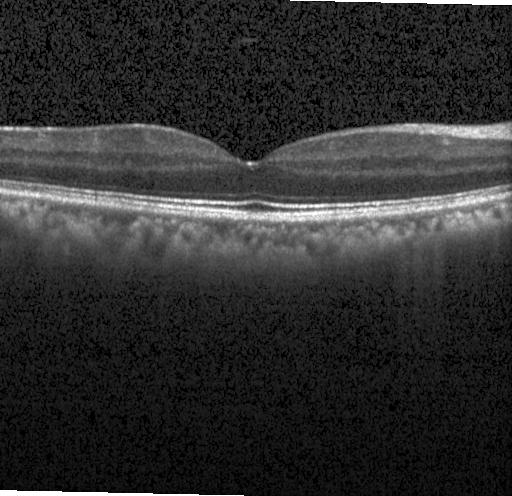

Optical coherence tomography scan · spectral-domain OCT · Heidelberg Spectralis OCT system.
Dx: no CNV, DME, or drusen.